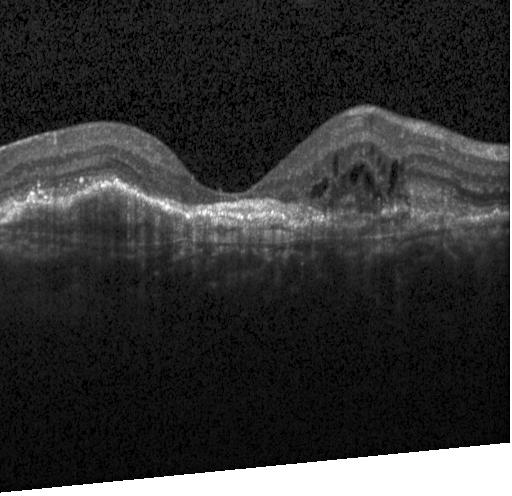
Macular scan, OCT line scan, spectral-domain optical coherence tomography
Assessment: a choroidal neovascular membrane.